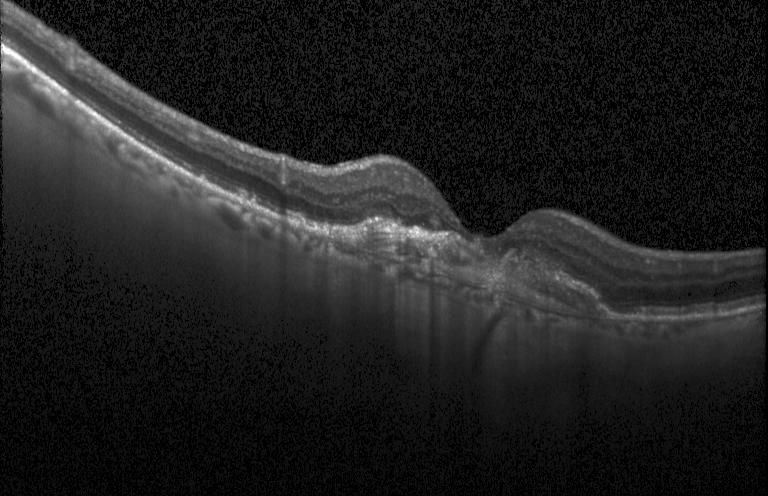 Macular OCT: choroidal neovascularization (CNV).